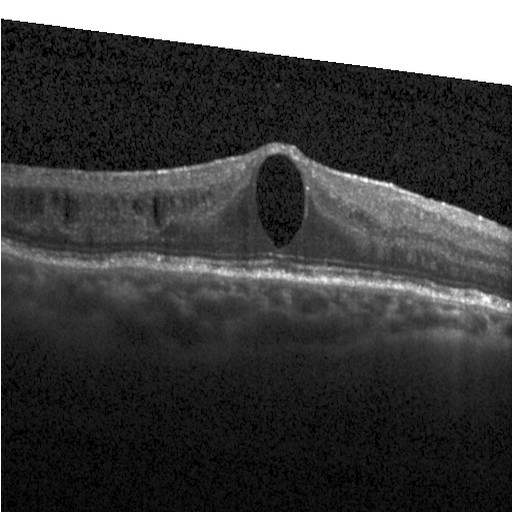 Spectral-domain optical coherence tomography. OCT B-scan.
Finding: diabetic macular edema (DME).